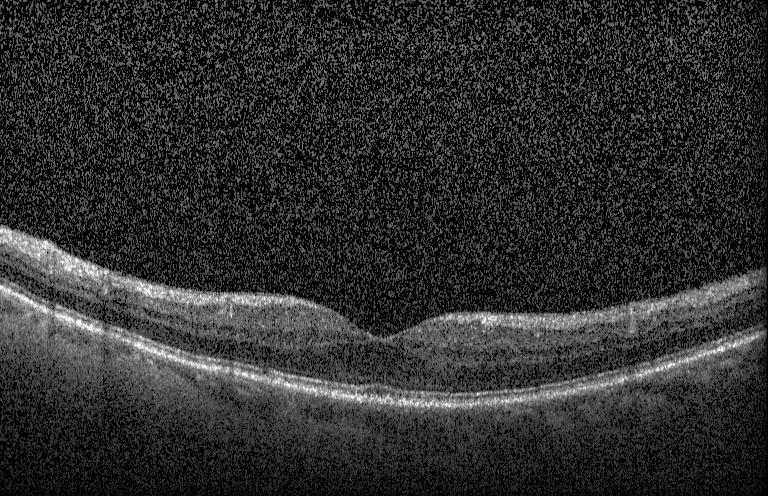

OCT line scan. Heidelberg Spectralis OCT system. SD-OCT. Horizontal scan through the fovea. Diagnosis: no choroidal neovascularization, diabetic macular edema, or drusen.